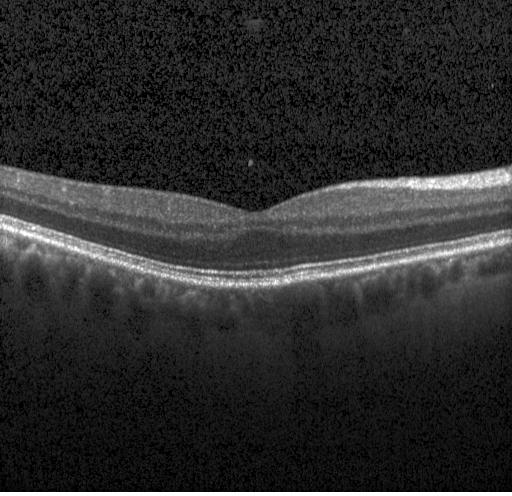 Retinal OCT cross-section; spectral-domain OCT — Diagnosis: no choroidal neovascularization, diabetic macular edema, or drusen.